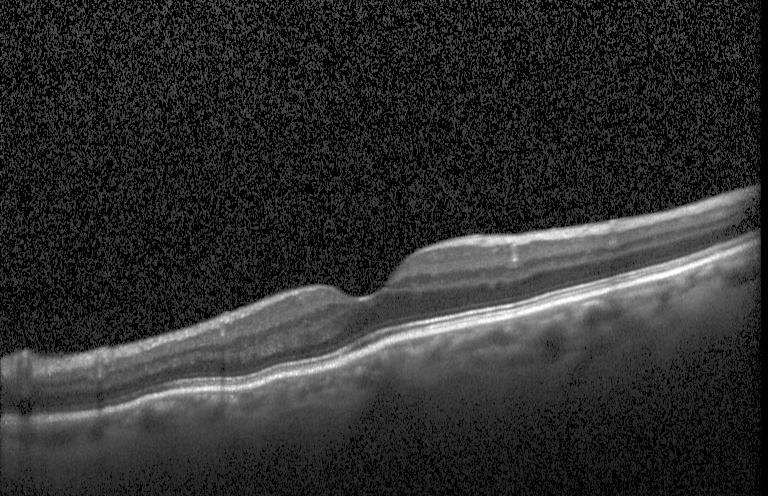

OCT B-scan. Heidelberg Spectralis. Spectral-domain OCT. Through the macula
Diagnosis: neither CNV, DME, nor drusen.